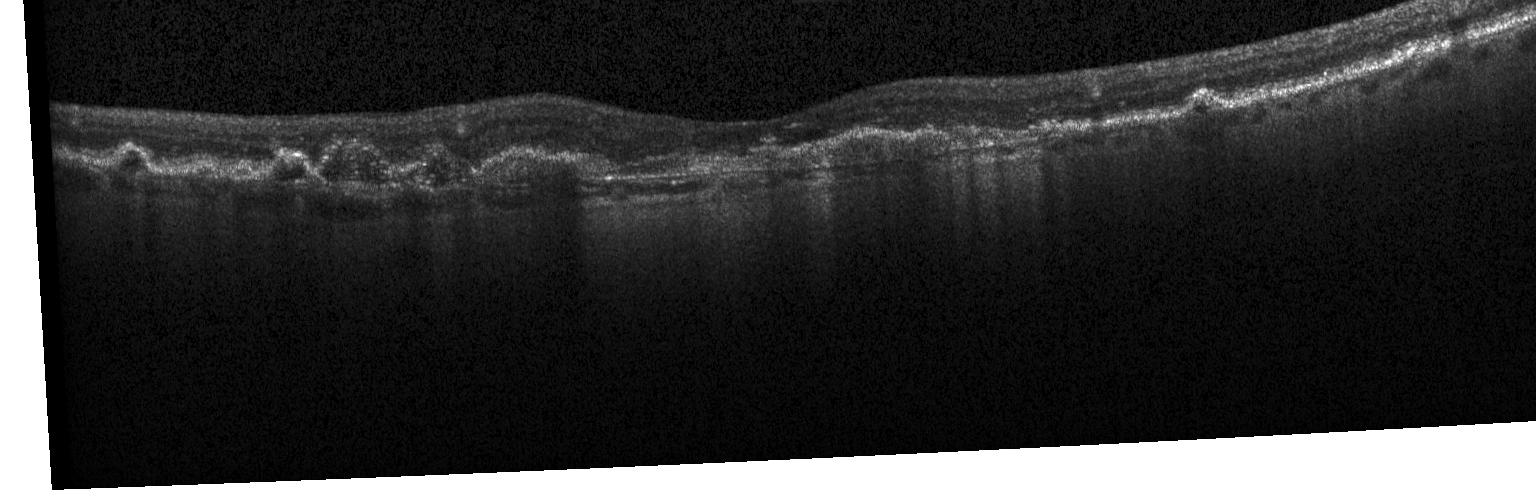

CNV.